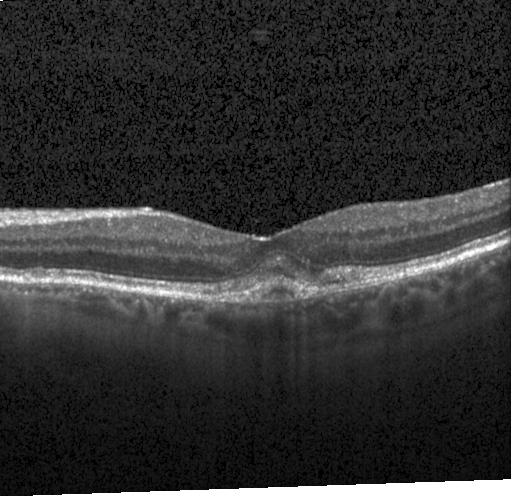
OCT B-scan · spectral-domain OCT
Impression: CNV.